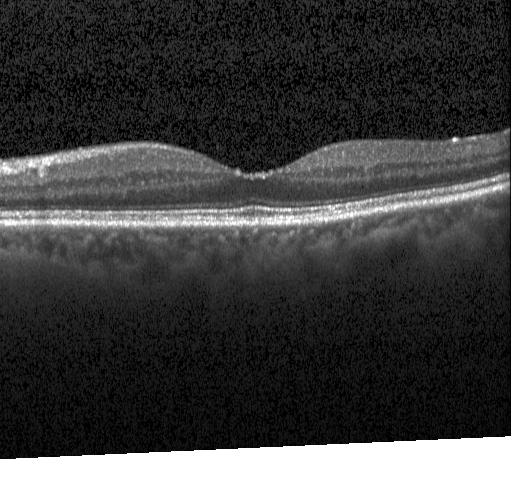 OCT finding: no CNV, no DME, and no drusen.